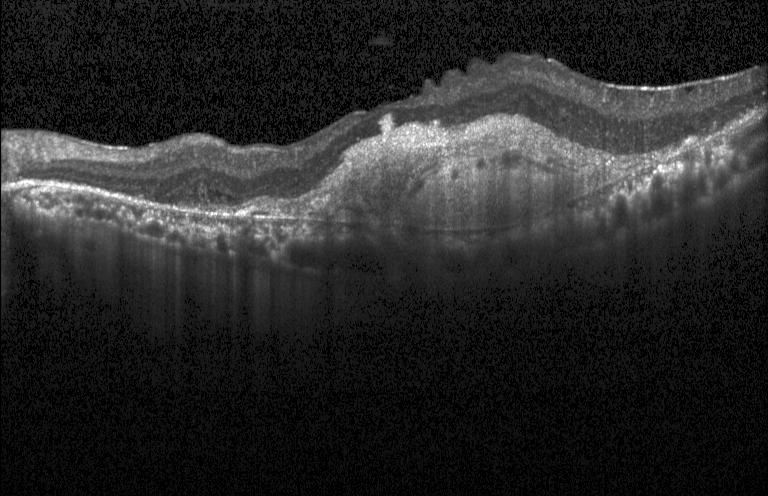
Diagnosis: a choroidal neovascular membrane.